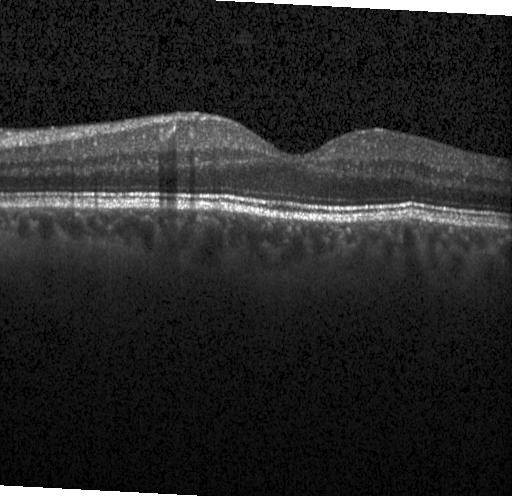
Instrument: Heidelberg Spectralis, fovea-centered, optical coherence tomography scan.
The scan shows no evidence of CNV, DME, or drusen.